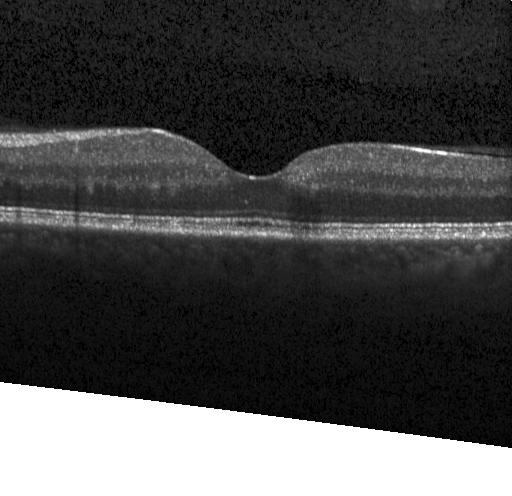
Dx: no evidence of choroidal neovascularization, diabetic macular edema, or drusen.